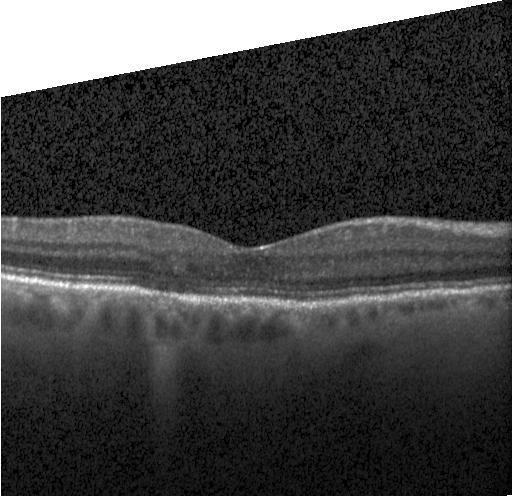

OCT line scan — Dx: no evidence of choroidal neovascularization, diabetic macular edema, or drusen.